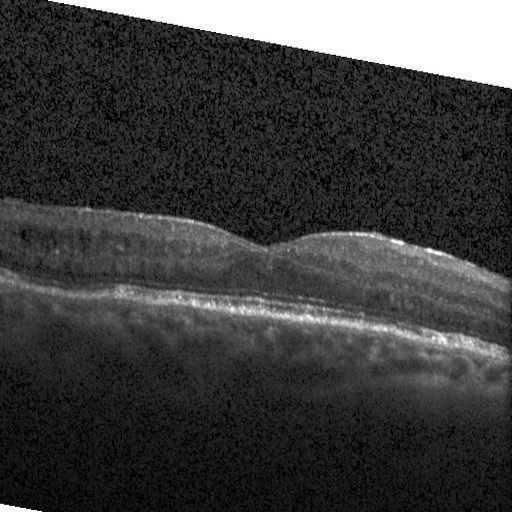
Retinal OCT cross-section · fovea-centered. This B-scan demonstrates diabetic macular edema (DME).